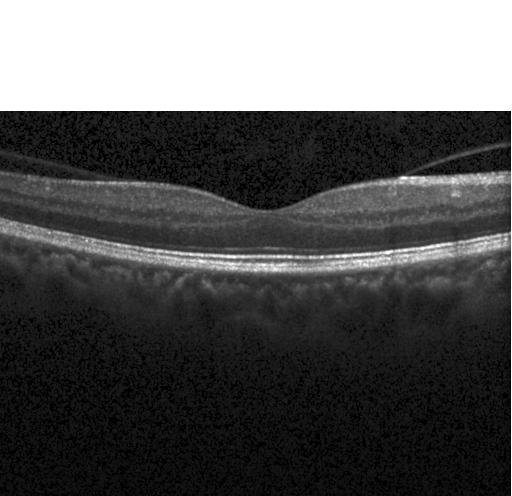

Optical coherence tomography scan.
Diagnosis: no choroidal neovascularization, no diabetic macular edema, and no drusen.